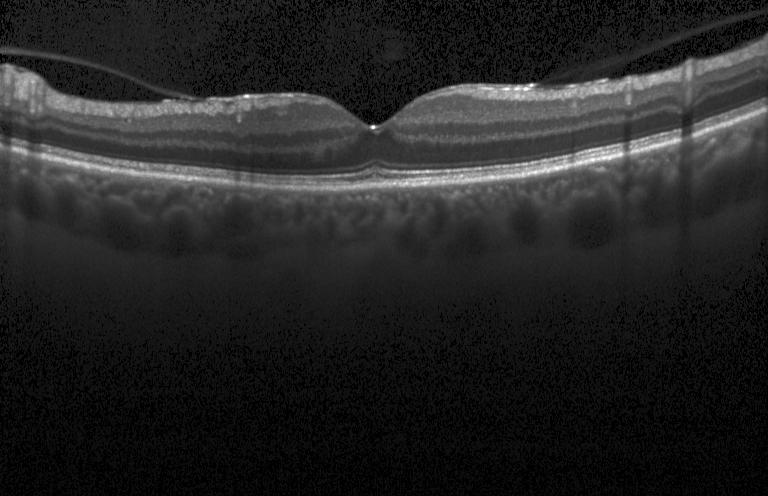
OCT scan showing no choroidal neovascularization, diabetic macular edema, or drusen.